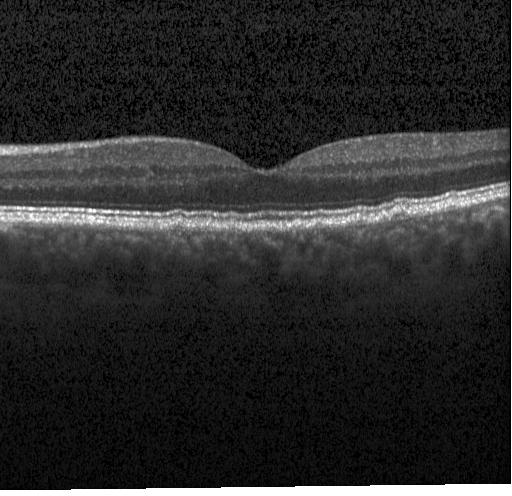
Retinal OCT B-scan · Heidelberg Spectralis OCT system
Macular OCT: multiple drusen.